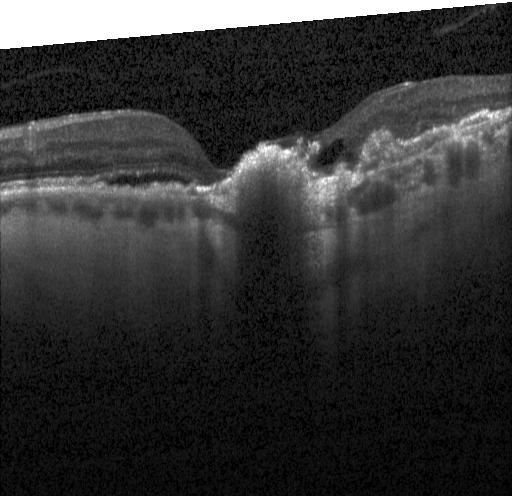 OCT scan showing choroidal neovascularization.